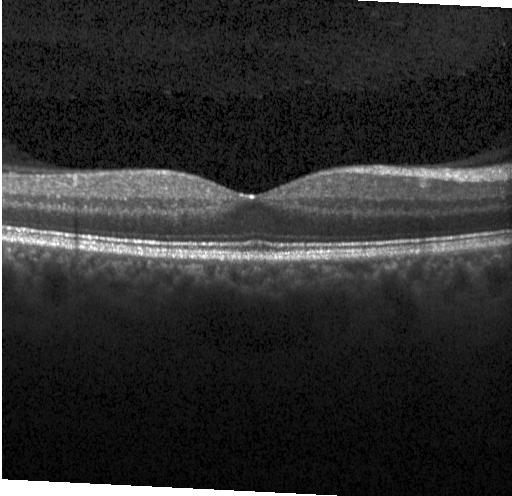 Macular OCT demonstrating no evidence of choroidal neovascularization, diabetic macular edema, or drusen.